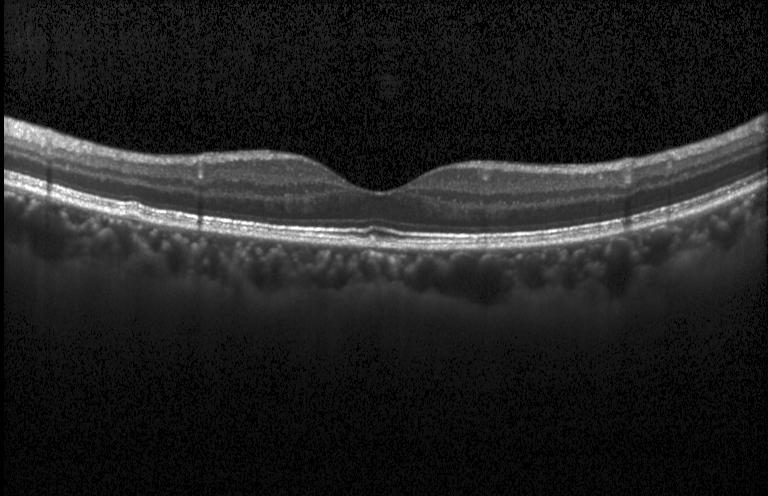

No CNV, no DME, and no drusen.